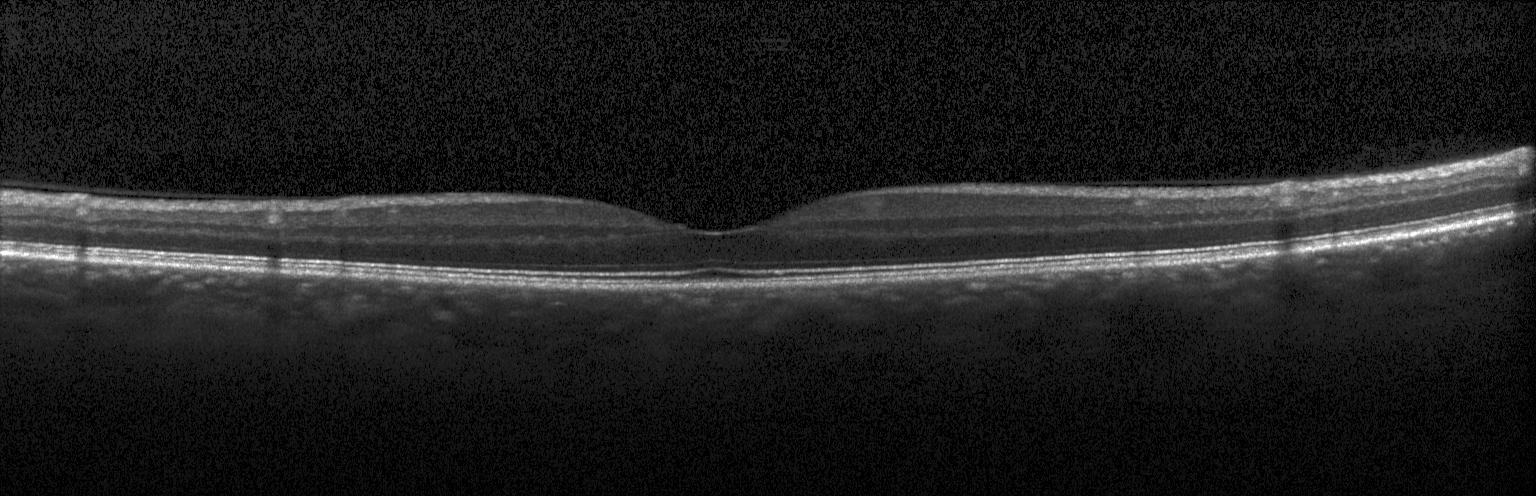 OCT B-scan showing no evidence of CNV, DME, or drusen.